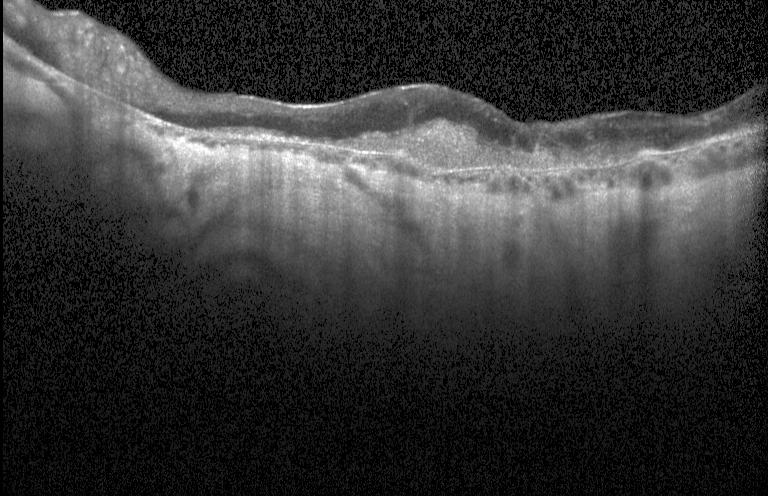

Spectral-domain OCT B-scan: a choroidal neovascular membrane.